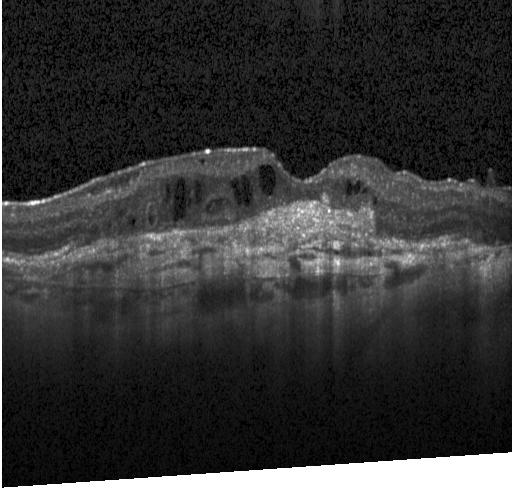 Optical coherence tomography B-scan. Finding: CNV.